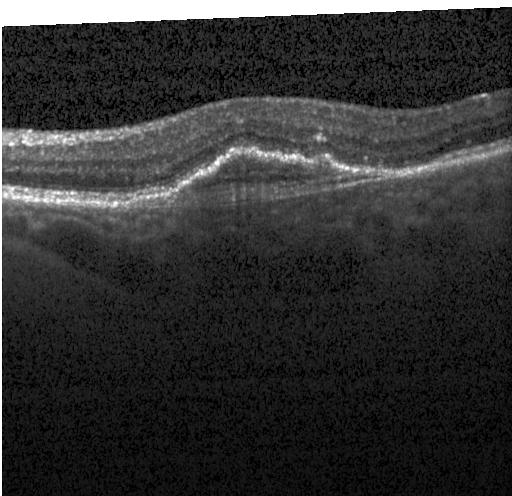
Diagnosis: CNV.